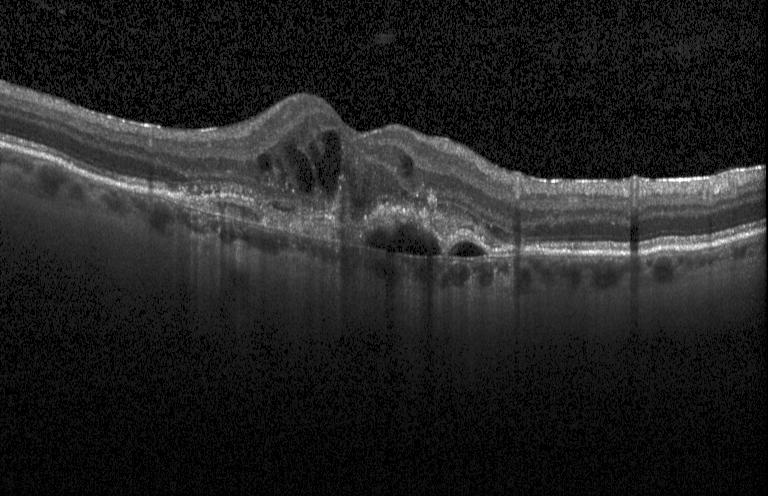
OCT line scan. Choroidal neovascularization.